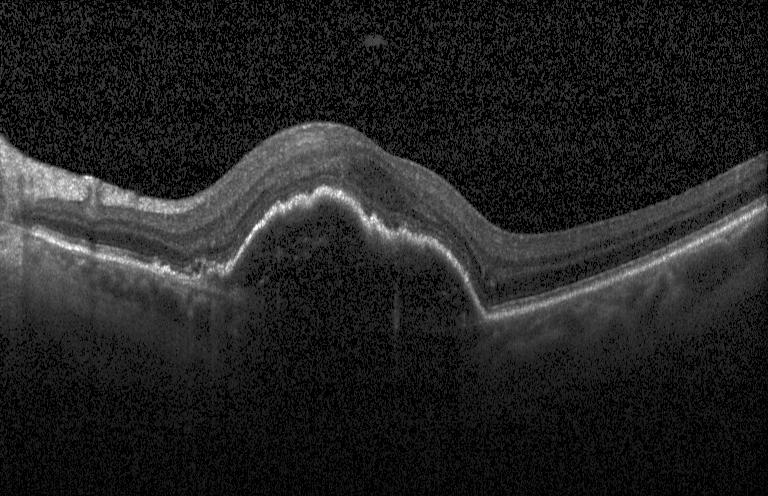

Macular scan. OCT line scan — The scan shows choroidal neovascularization (CNV).